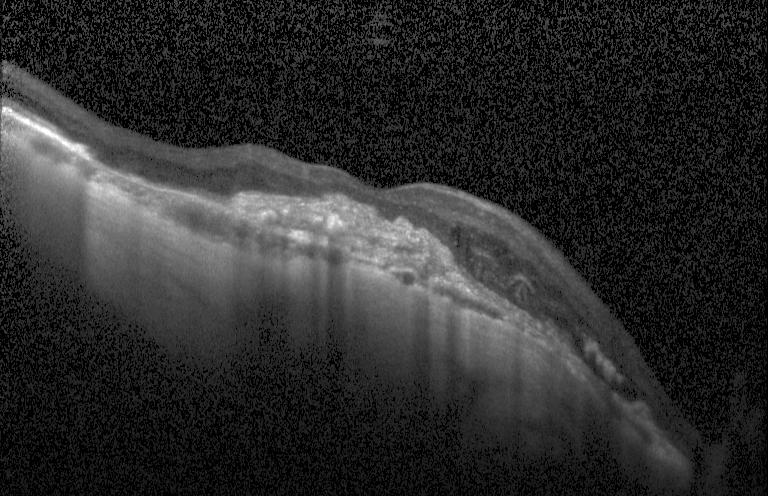 OCT B-scan · spectral-domain OCT · Heidelberg Spectralis · horizontal scan through the fovea.
Diagnosis: choroidal neovascularization (CNV).